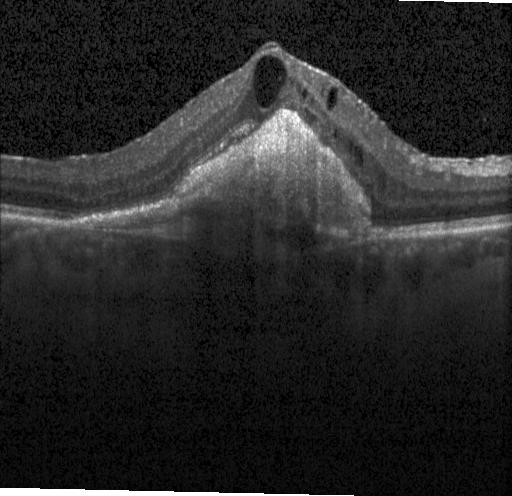
Retinal OCT cross-section. Heidelberg Spectralis. Spectral-domain OCT. Impression: choroidal neovascularization.